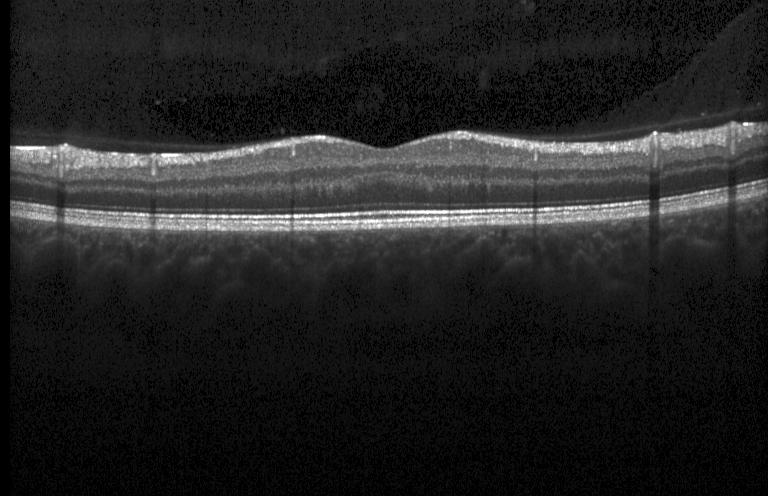 Macular scan. Optical coherence tomography B-scan. This B-scan demonstrates no choroidal neovascularization, no diabetic macular edema, and no drusen.